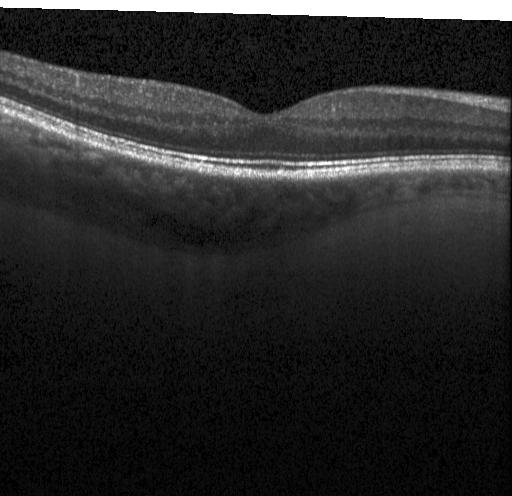

Acquired on a Heidelberg Spectralis; macular scan; retinal OCT cross-section.
Diagnosis: no choroidal neovascularization, diabetic macular edema, or drusen.